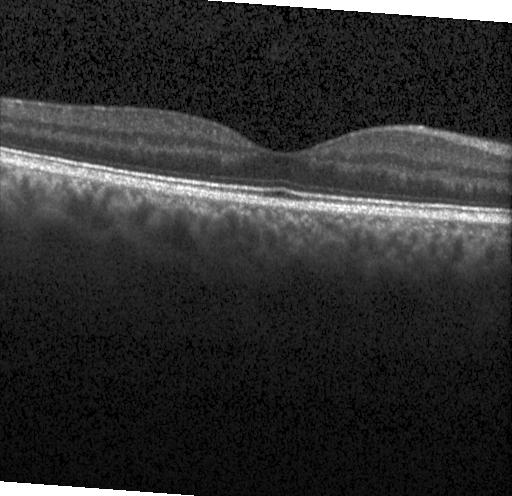

OCT line scan.
Impression: neither choroidal neovascularization, diabetic macular edema, nor drusen.